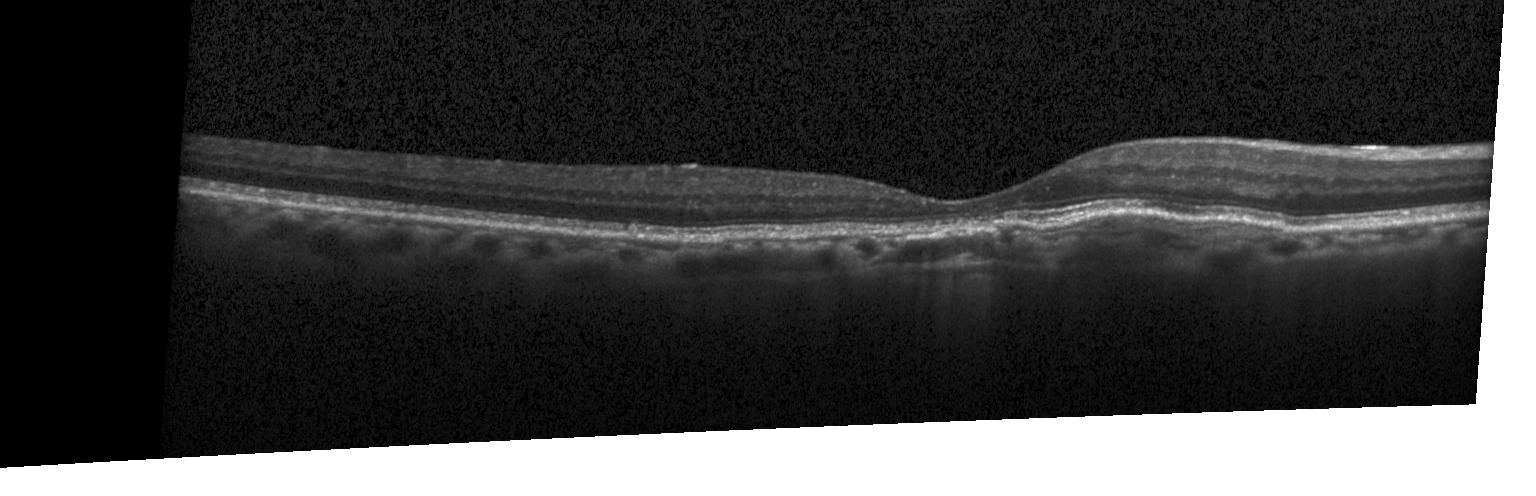

Spectral-domain OCT, acquired on a Heidelberg Spectralis, horizontal scan through the fovea, optical coherence tomography B-scan — OCT finding: a choroidal neovascular membrane.